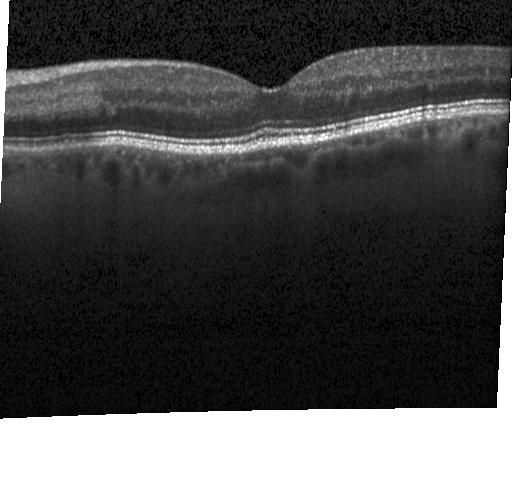

Optical coherence tomography B-scan, Heidelberg Spectralis OCT system.
Dx: no choroidal neovascularization, diabetic macular edema, or drusen.